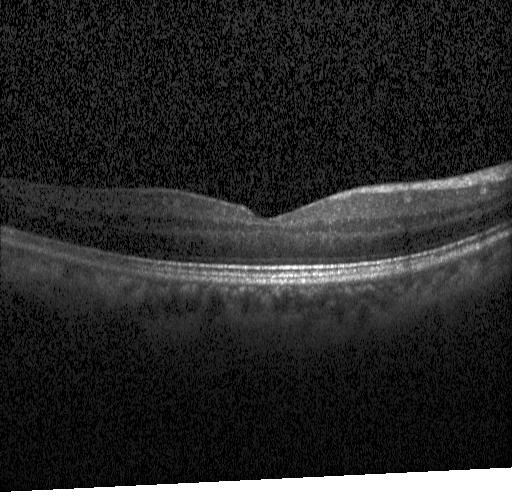 Centered on the fovea · Heidelberg Spectralis · optical coherence tomography B-scan · spectral-domain OCT. Finding: neither CNV, DME, nor drusen.